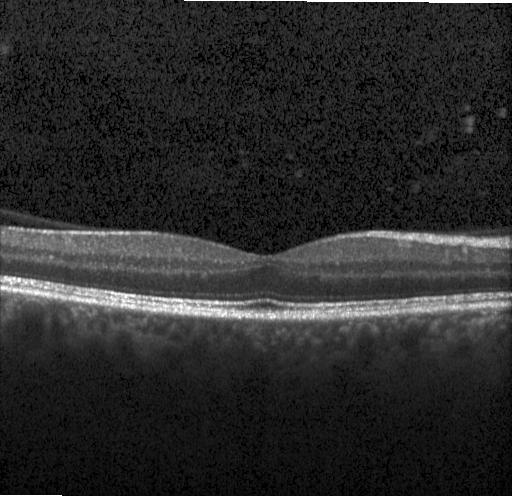
Optical coherence tomography scan, macular scan, spectral-domain OCT, Heidelberg Spectralis — Diagnosis: neither CNV, DME, nor drusen.